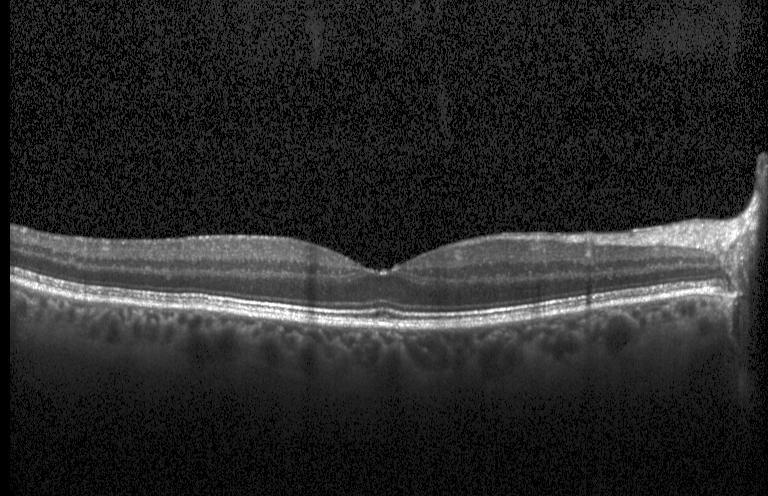
The scan shows no choroidal neovascularization, diabetic macular edema, or drusen.